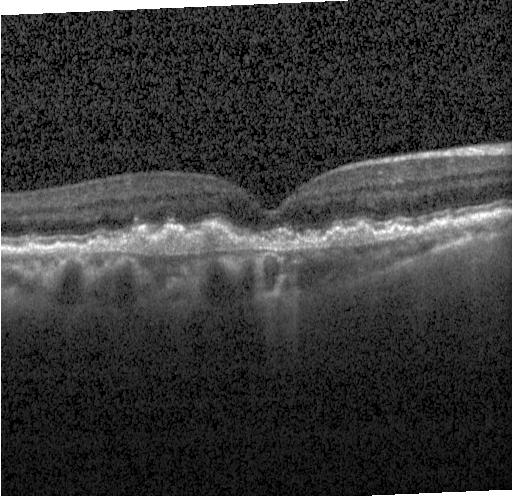

Spectral-domain OCT · optical coherence tomography scan · through the macula · Heidelberg Spectralis
Finding: CNV.